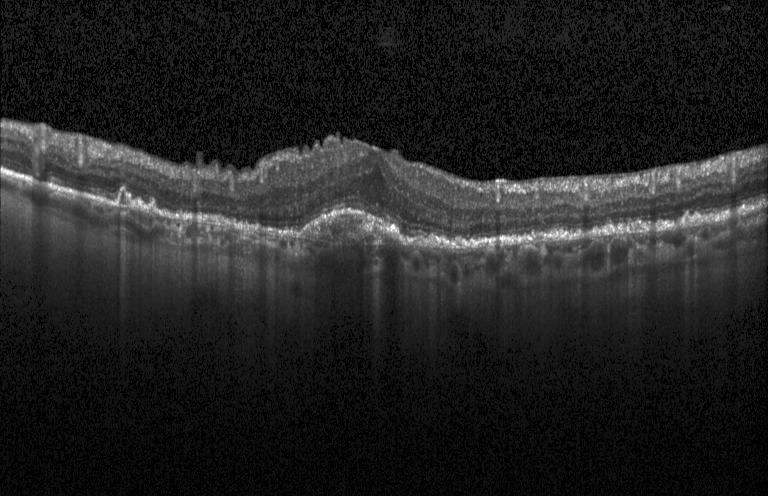
Retinal OCT cross-section
A choroidal neovascular membrane.